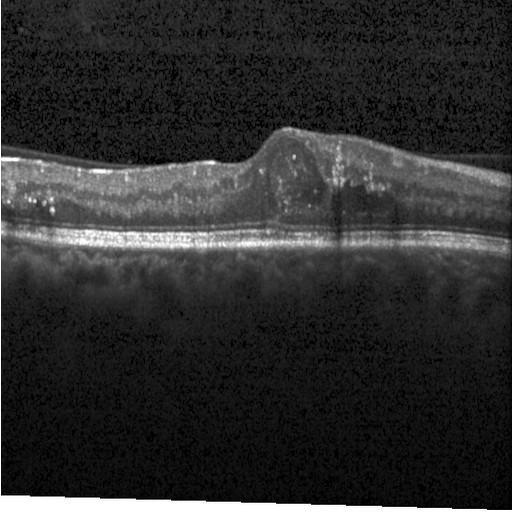

Optical coherence tomography scan
Impression: DME.